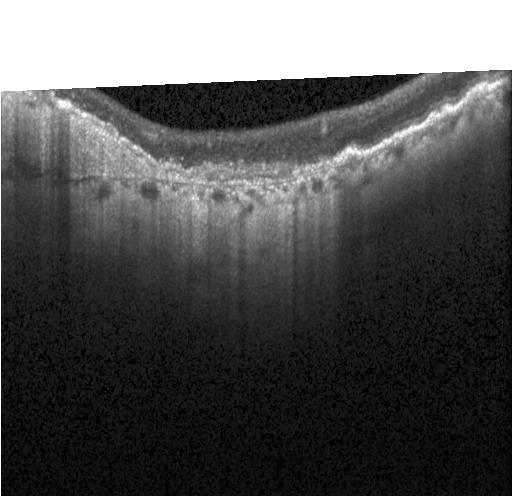

Impression: a choroidal neovascular membrane.